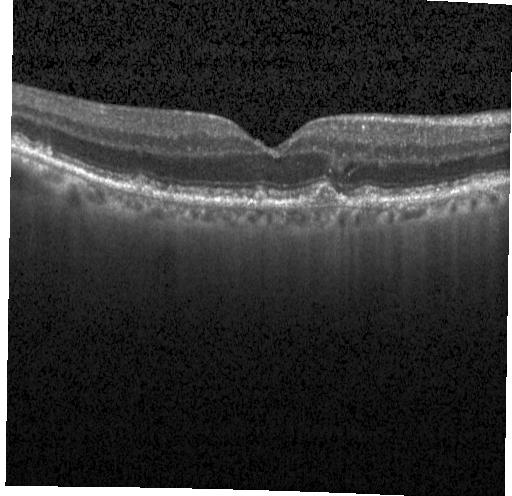

OCT B-scan — Assessment: multiple drusen.